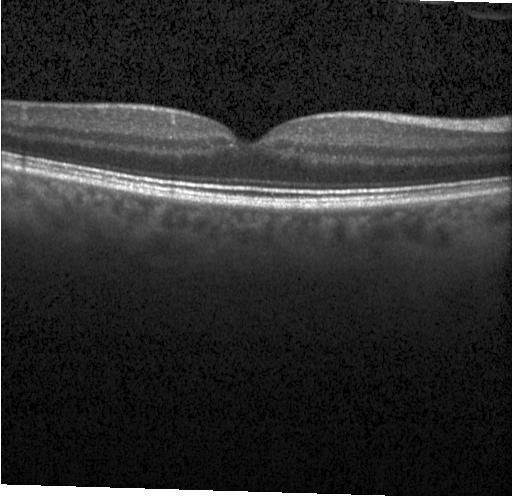
Retinal OCT cross-section · SD-OCT · centered on the fovea — Macular OCT: no evidence of CNV, DME, or drusen.